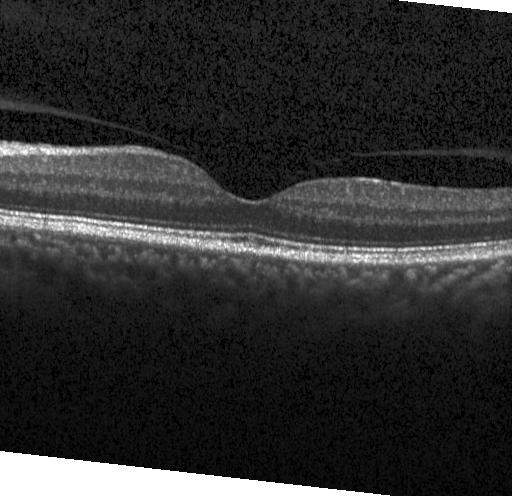
Optical coherence tomography scan; fovea-centered. Assessment: no evidence of choroidal neovascularization, diabetic macular edema, or drusen.